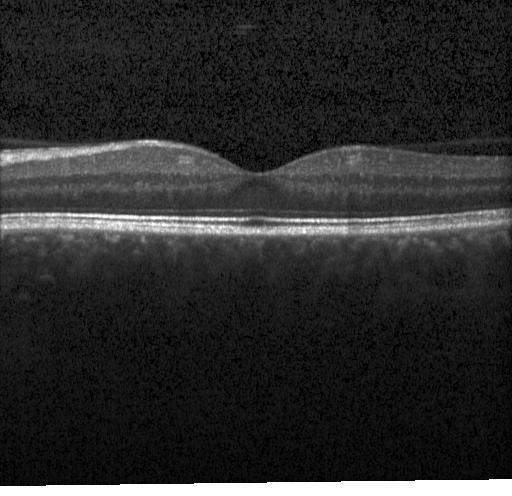

Finding: no CNV, DME, or drusen.